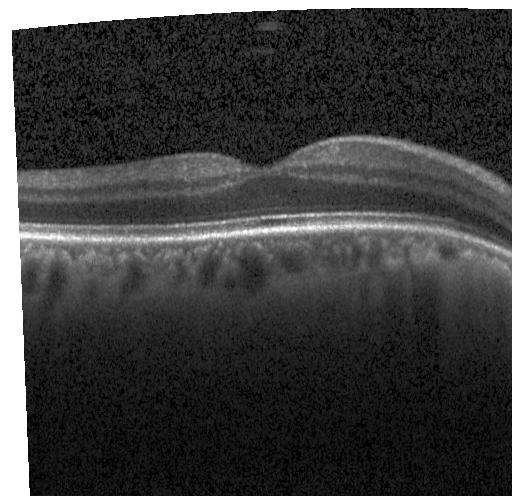
No evidence of choroidal neovascularization, diabetic macular edema, or drusen.